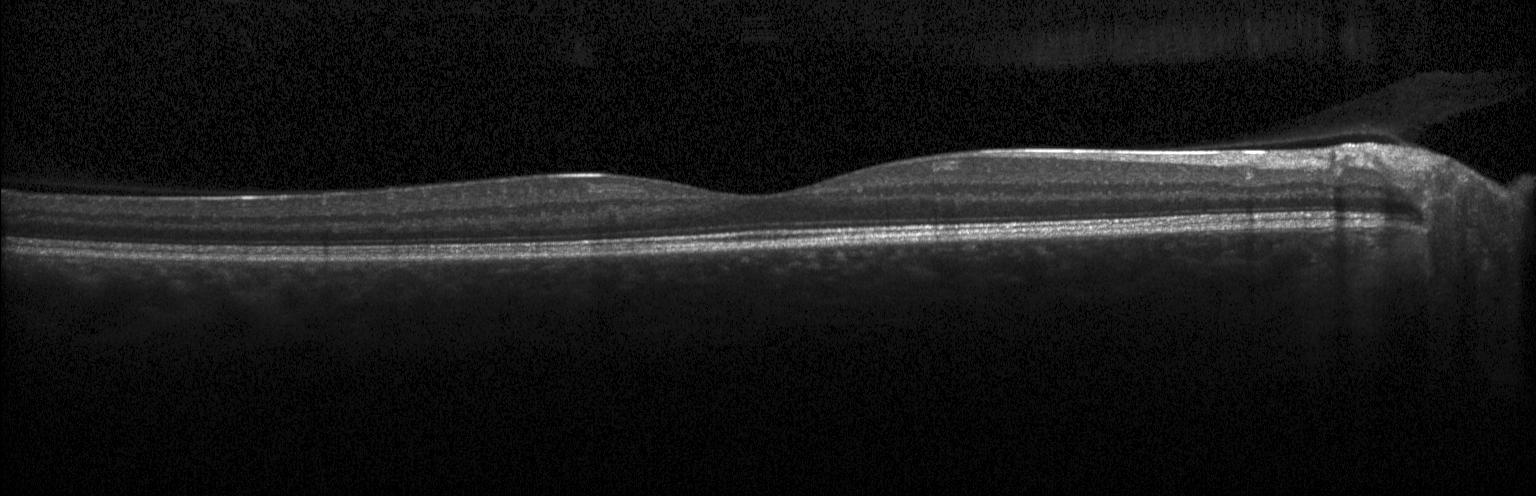

SD-OCT · Heidelberg Spectralis OCT system · macular scan · optical coherence tomography B-scan.
Dx: no evidence of CNV, DME, or drusen.